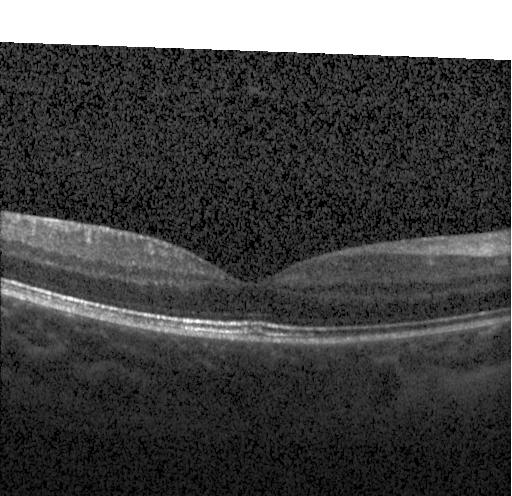

Retinal OCT cross-section showing no choroidal neovascularization, no diabetic macular edema, and no drusen.